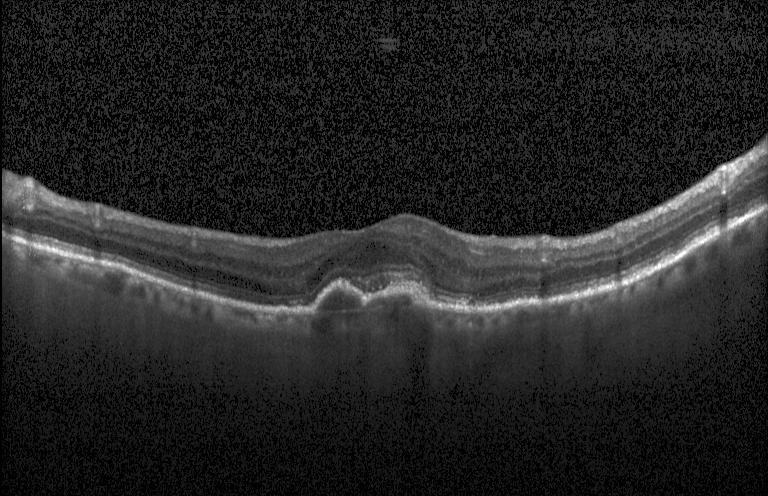
The scan shows a choroidal neovascular membrane.